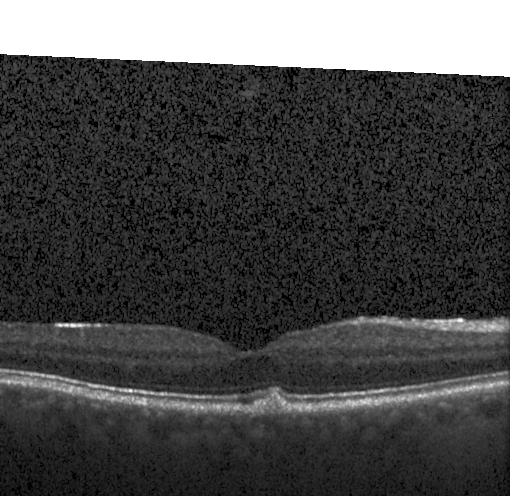
Through the macula, Heidelberg Spectralis OCT system, spectral-domain OCT, optical coherence tomography B-scan
Assessment: sub-RPE drusenoid deposits.